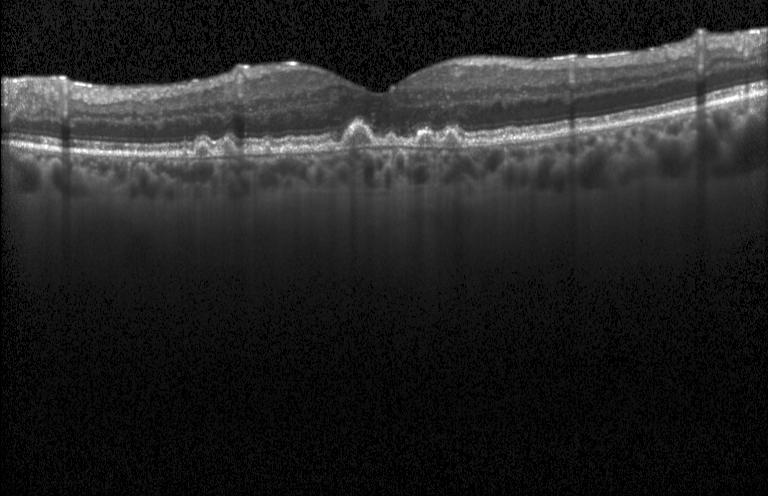
Centered on the fovea · spectral-domain optical coherence tomography · acquired on a Heidelberg Spectralis · OCT line scan. Finding: multiple drusen.